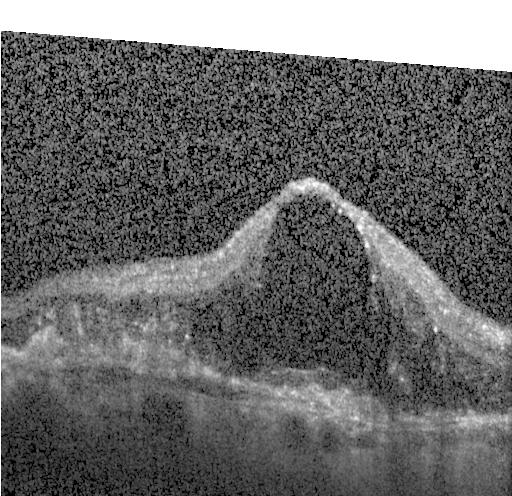
Assessment: CNV.